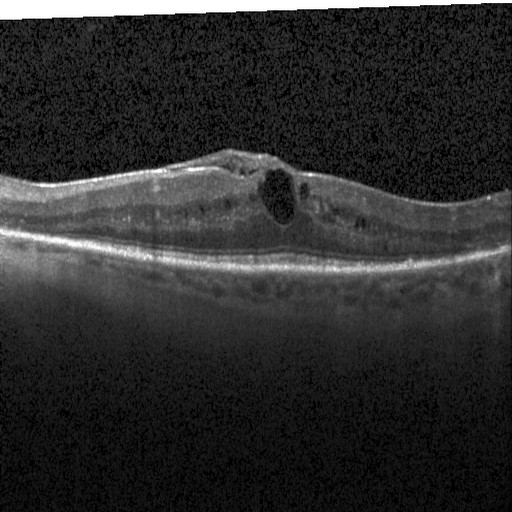

OCT finding: diabetic macular edema (DME).